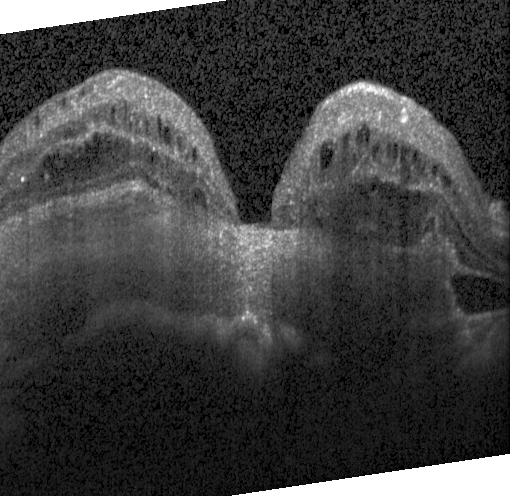

Spectral-domain OCT; through the macula; retinal OCT cross-section; instrument: Heidelberg Spectralis.
The scan shows choroidal neovascularization.